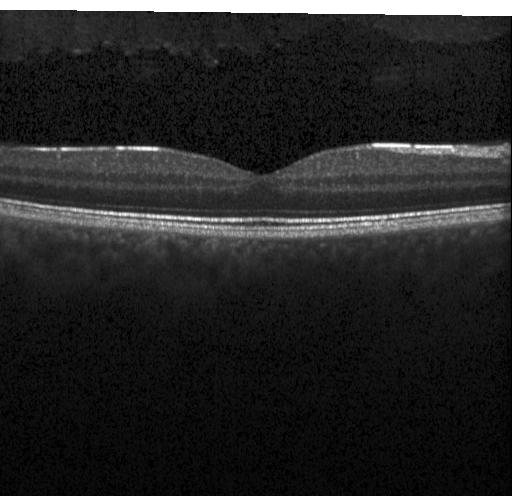

Instrument: Heidelberg Spectralis; OCT line scan; SD-OCT
Diagnosis: neither CNV, DME, nor drusen.